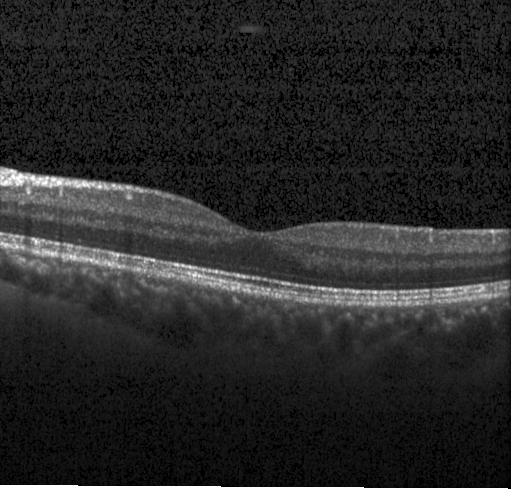

Diagnosis: no choroidal neovascularization, diabetic macular edema, or drusen.